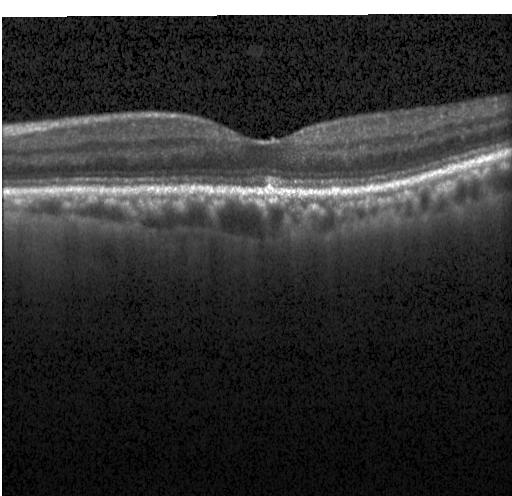 Spectral-domain OCT B-scan: neither CNV, DME, nor drusen.